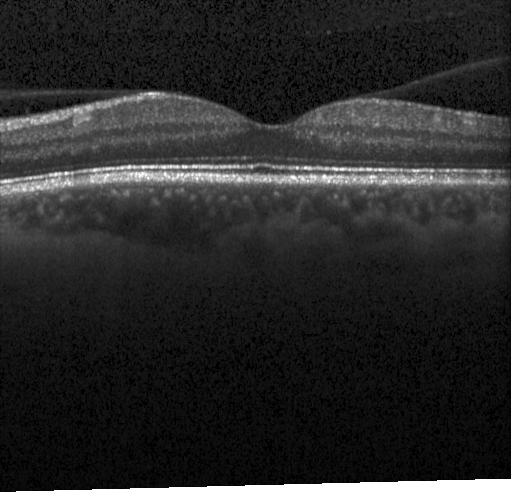
Diagnosis: no evidence of choroidal neovascularization, diabetic macular edema, or drusen.